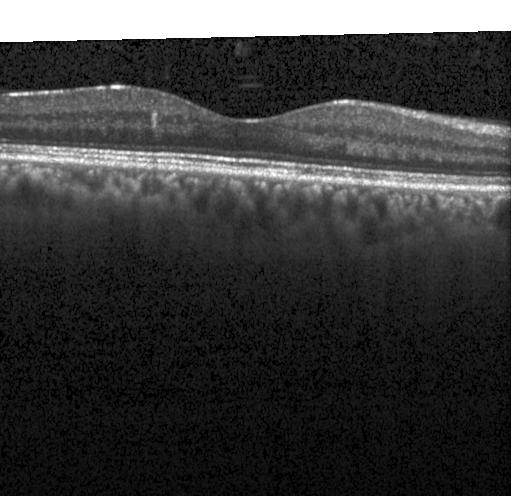
Macular OCT demonstrating neither choroidal neovascularization, diabetic macular edema, nor drusen.